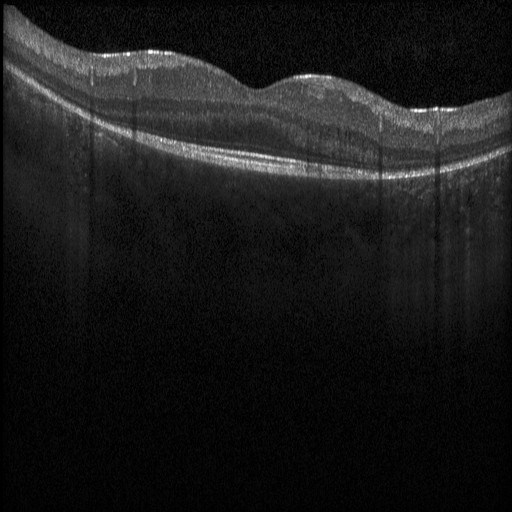 Acquired on a Heidelberg Spectralis, retinal OCT B-scan, macular scan, SD-OCT — Diagnosis: diabetic macular edema (DME).